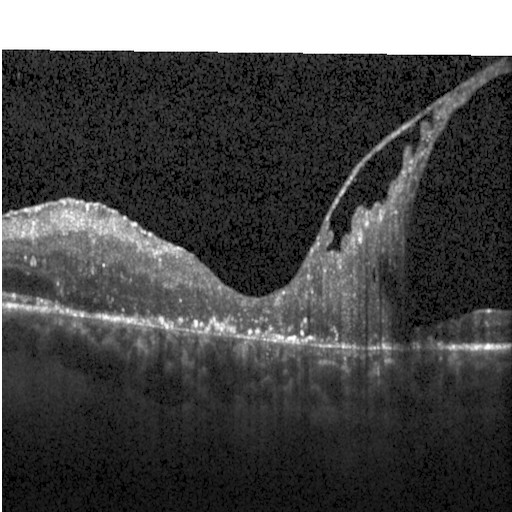
Macular OCT demonstrating diabetic macular edema (DME).